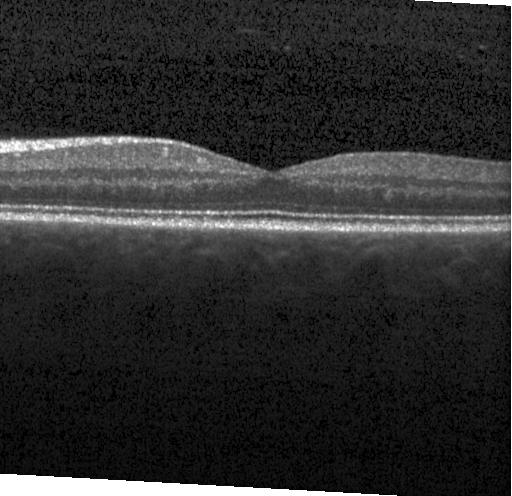 OCT scan showing neither choroidal neovascularization, diabetic macular edema, nor drusen.